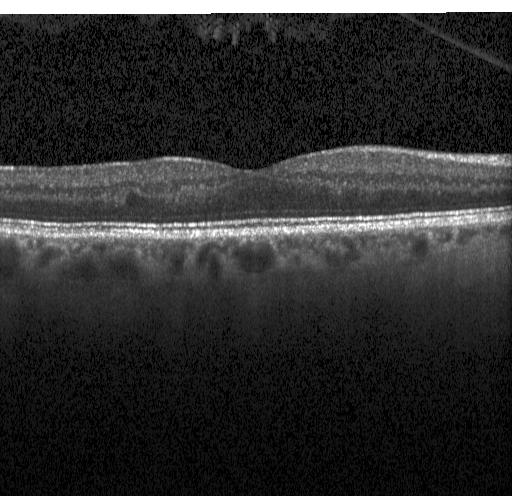
Instrument: Heidelberg Spectralis · OCT B-scan · spectral-domain OCT
OCT finding: neither choroidal neovascularization, diabetic macular edema, nor drusen.